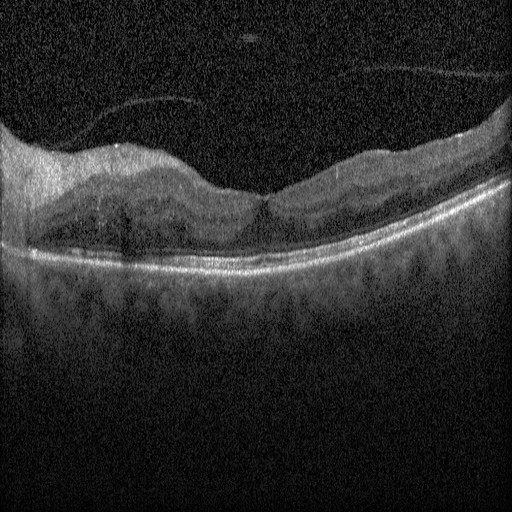

Dx: diabetic macular edema.